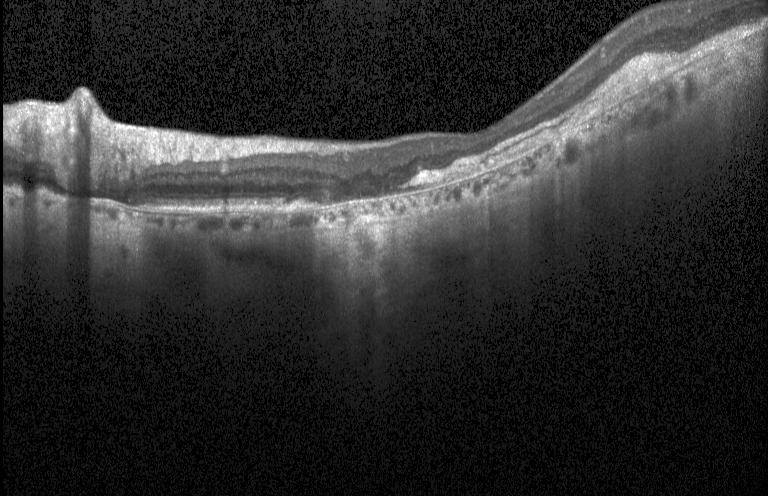 Spectral-domain OCT. Optical coherence tomography B-scan
Finding: a choroidal neovascular membrane.